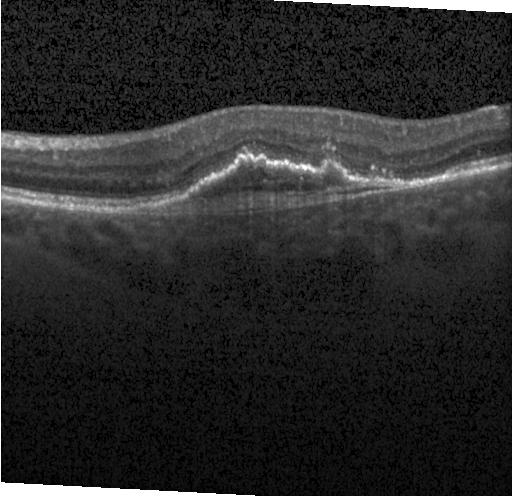 Macular OCT: a choroidal neovascular membrane.